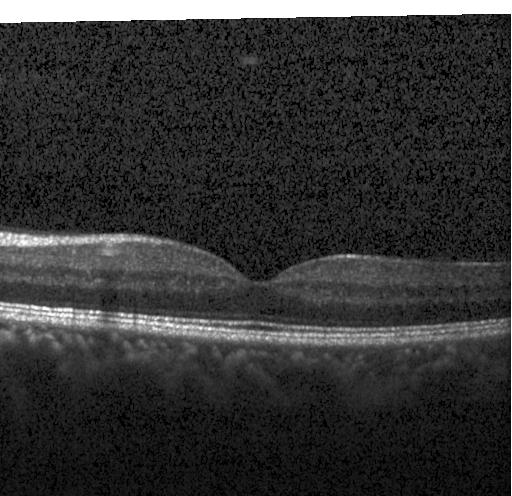
OCT scan showing no evidence of choroidal neovascularization, diabetic macular edema, or drusen.